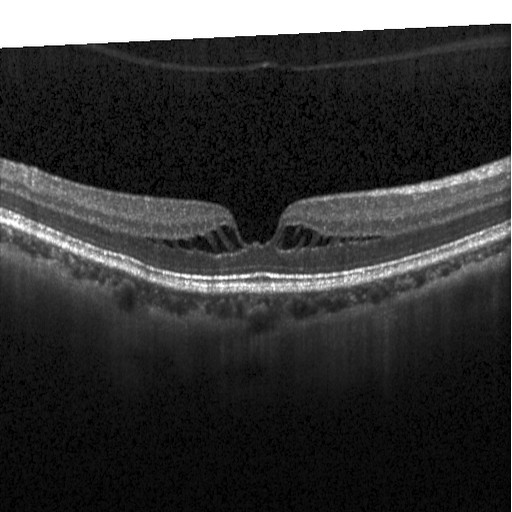
Assessment: diabetic macular edema.